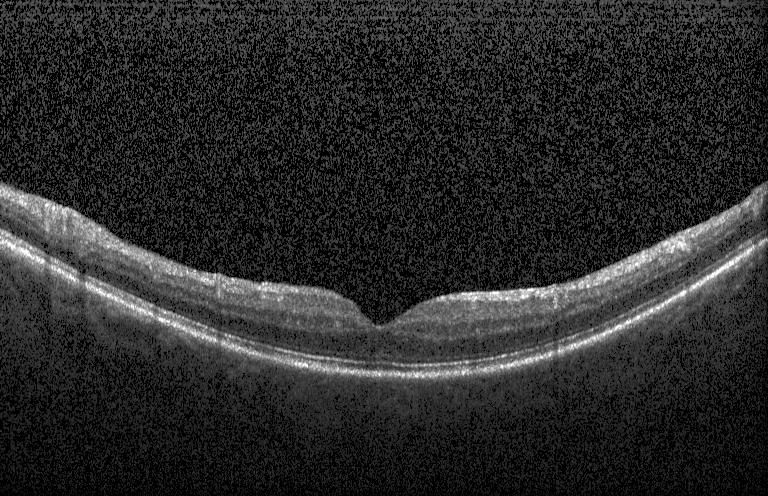
Macular scan. Optical coherence tomography scan. The scan shows no choroidal neovascularization, diabetic macular edema, or drusen.